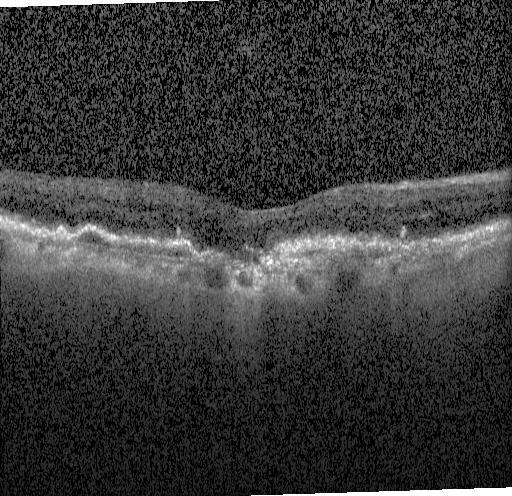
Through the macula; optical coherence tomography scan
This B-scan demonstrates choroidal neovascularization.